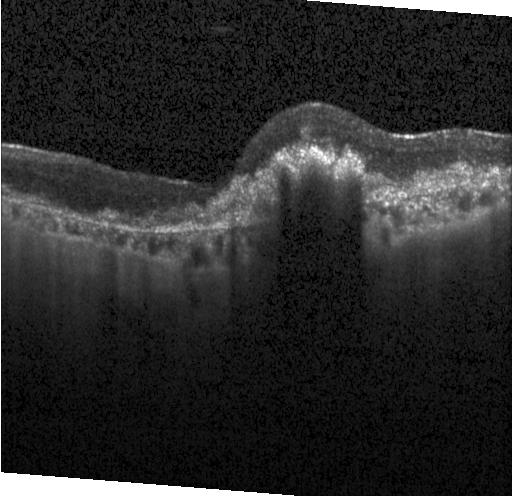
Fovea-centered; spectral-domain OCT; Heidelberg Spectralis; optical coherence tomography B-scan. Assessment: a choroidal neovascular membrane.